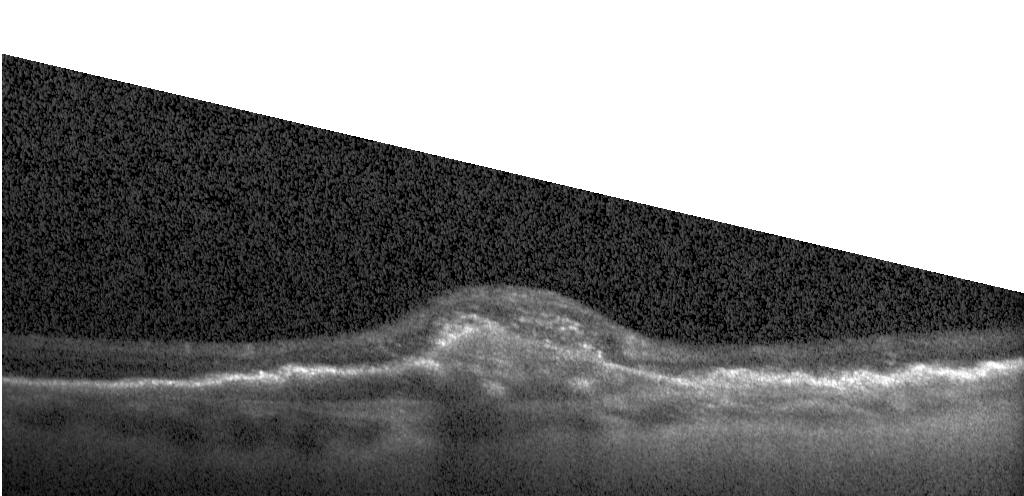

The scan shows choroidal neovascularization (CNV).